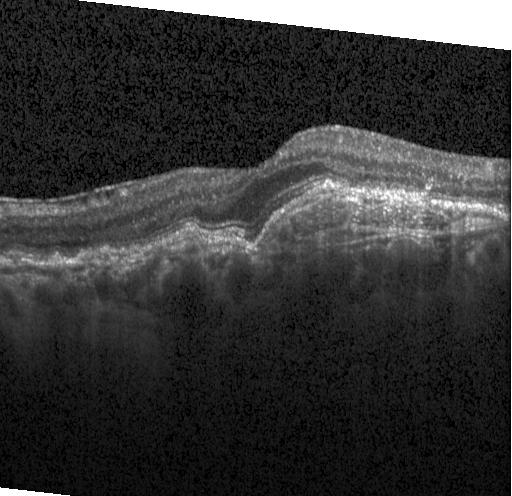

Retinal OCT B-scan. Spectral-domain OCT. Heidelberg Spectralis. Horizontal scan through the fovea.
The scan shows a choroidal neovascular membrane.